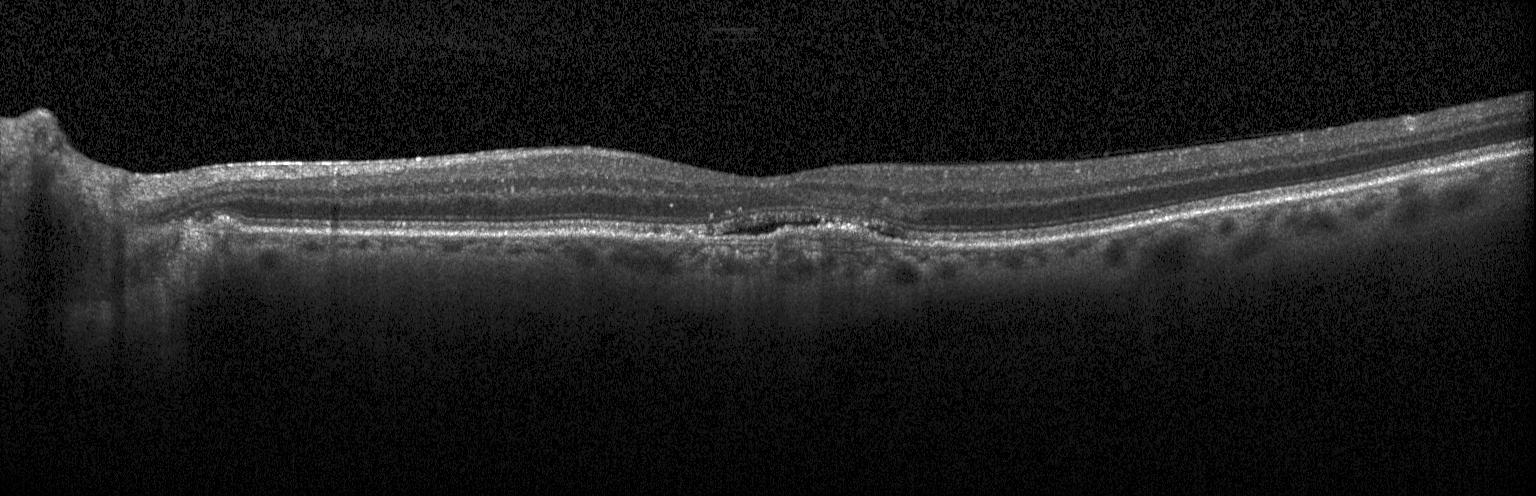 Finding: CNV.